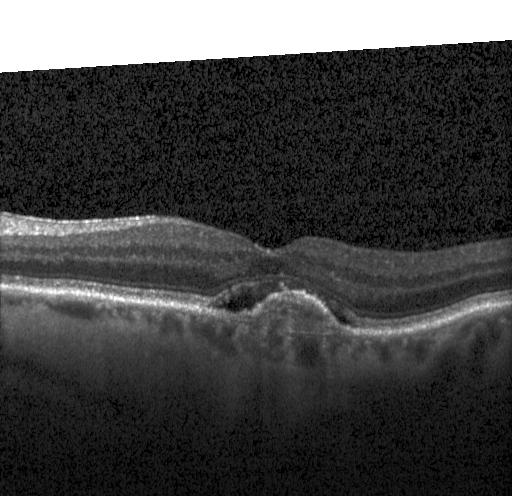 Instrument: Heidelberg Spectralis; retinal OCT B-scan; horizontal scan through the fovea.
This B-scan demonstrates a choroidal neovascular membrane.